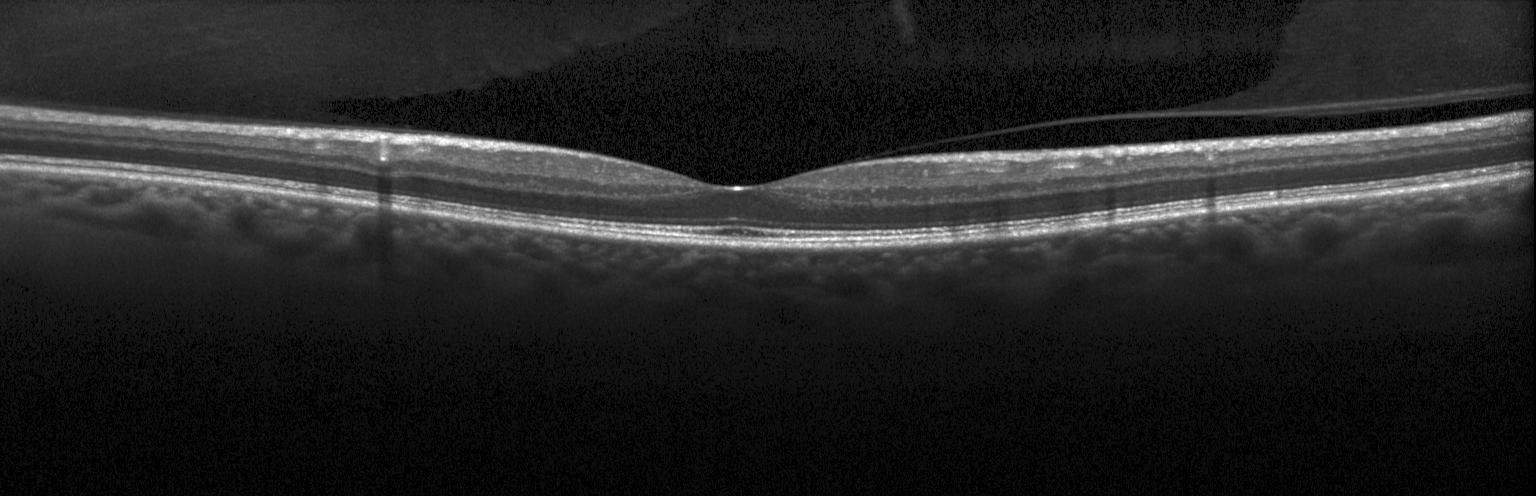

Acquired on a Heidelberg Spectralis, optical coherence tomography scan.
Diagnosis: no choroidal neovascularization, no diabetic macular edema, and no drusen.